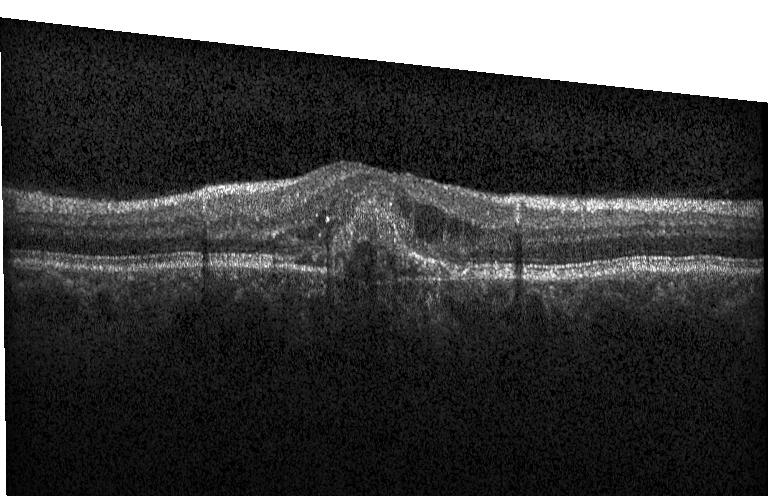
Heidelberg Spectralis, horizontal scan through the fovea, retinal OCT cross-section — Impression: a choroidal neovascular membrane.